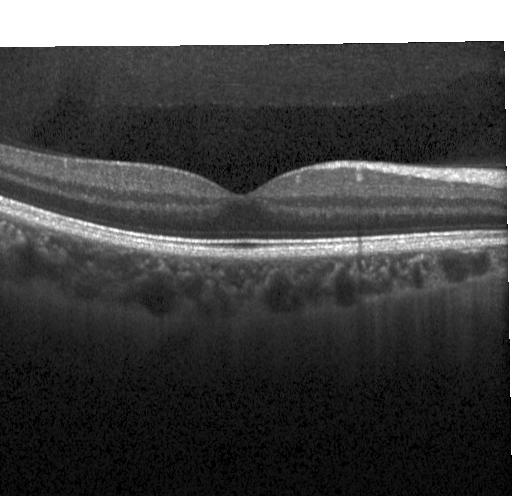

Optical coherence tomography B-scan — Impression: no evidence of choroidal neovascularization, diabetic macular edema, or drusen.